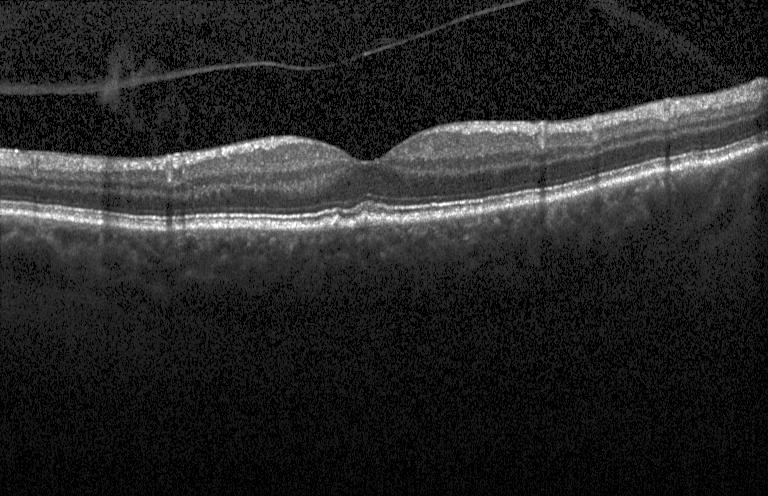 OCT line scan. Fovea-centered.
Dx: multiple drusen.